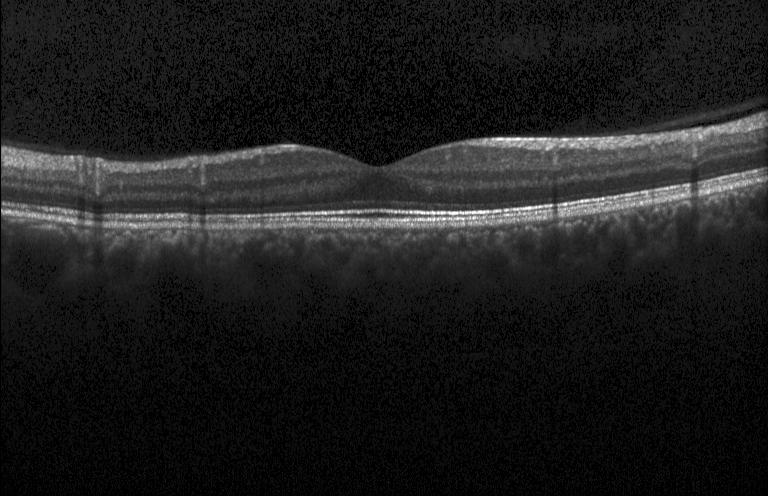

Neither choroidal neovascularization, diabetic macular edema, nor drusen.